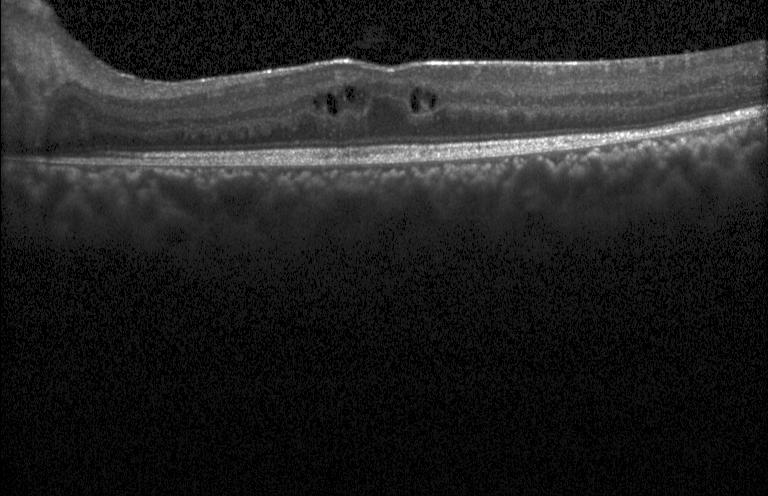 Impression: diabetic macular edema (DME).